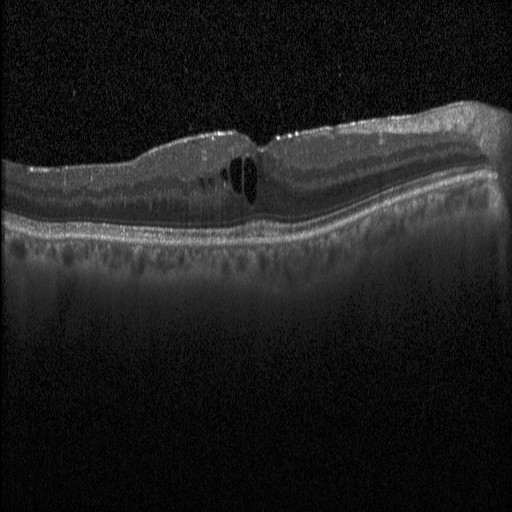
Retinal OCT cross-section showing DME.